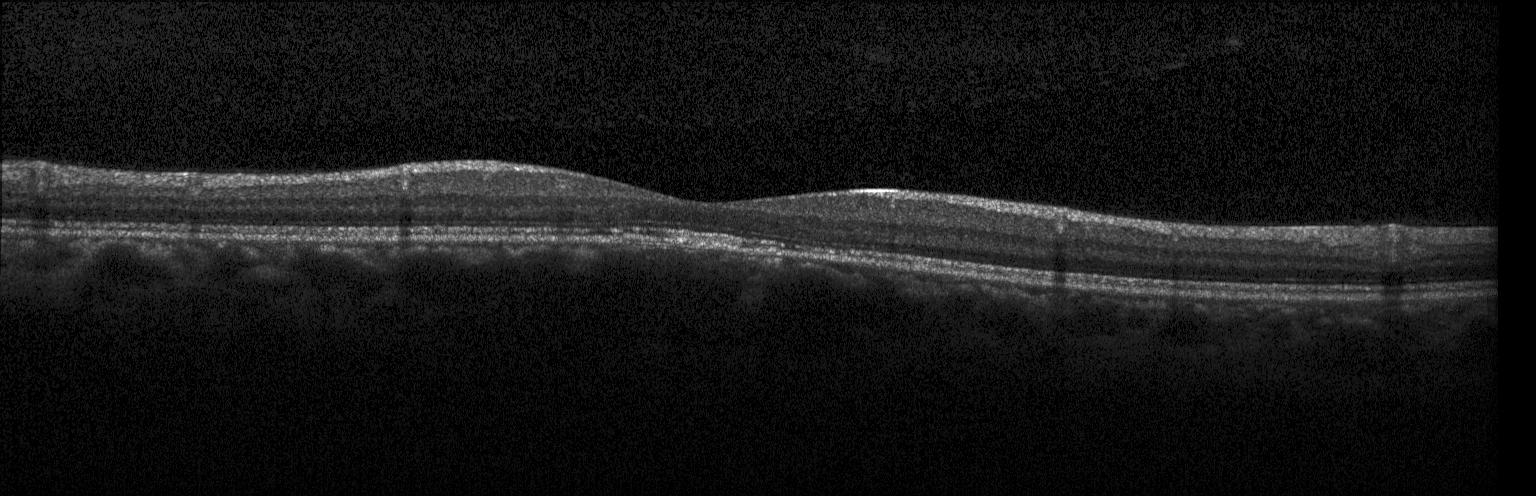 OCT B-scan showing no CNV, DME, or drusen.